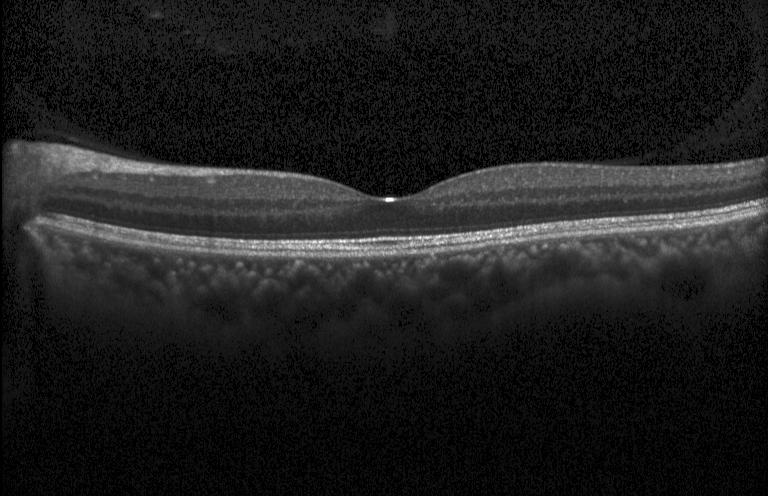
Horizontal scan through the fovea; optical coherence tomography B-scan; instrument: Heidelberg Spectralis.
Macular OCT: no choroidal neovascularization, no diabetic macular edema, and no drusen.